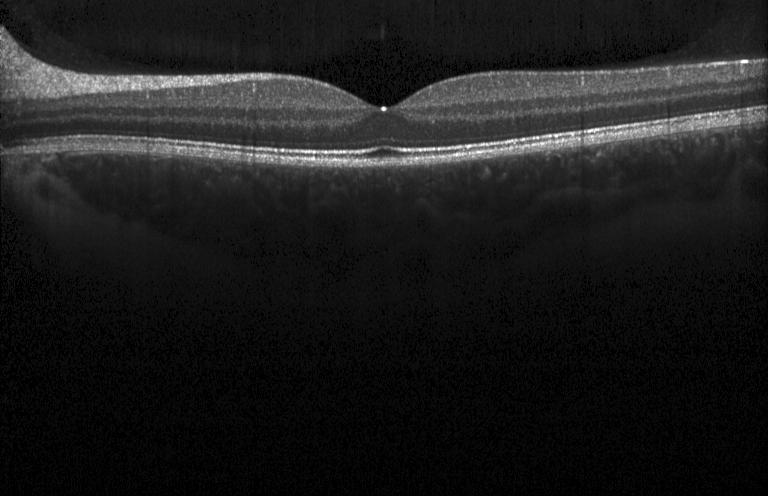 This B-scan demonstrates neither choroidal neovascularization, diabetic macular edema, nor drusen.